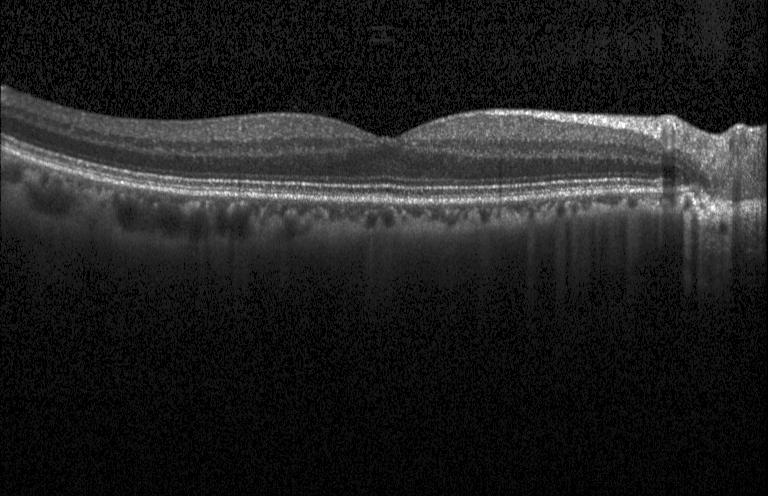 Centered on the fovea; Heidelberg Spectralis OCT system; optical coherence tomography scan; SD-OCT
Finding: no evidence of choroidal neovascularization, diabetic macular edema, or drusen.